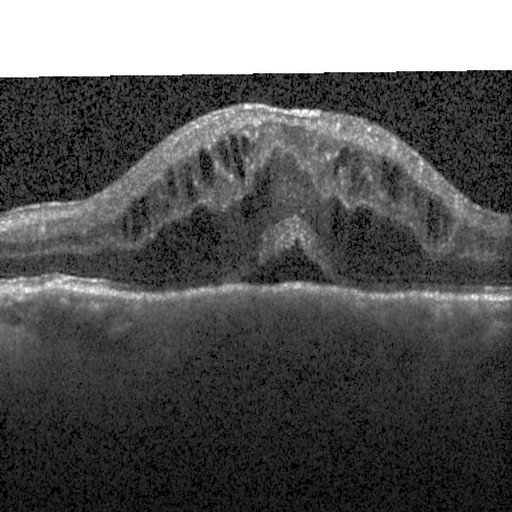
Retinal OCT cross-section — Finding: diabetic macular edema.